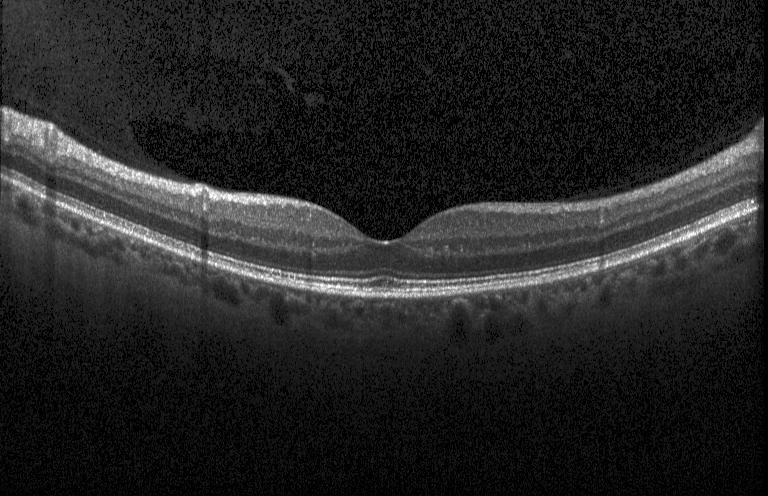
Finding: no evidence of choroidal neovascularization, diabetic macular edema, or drusen.